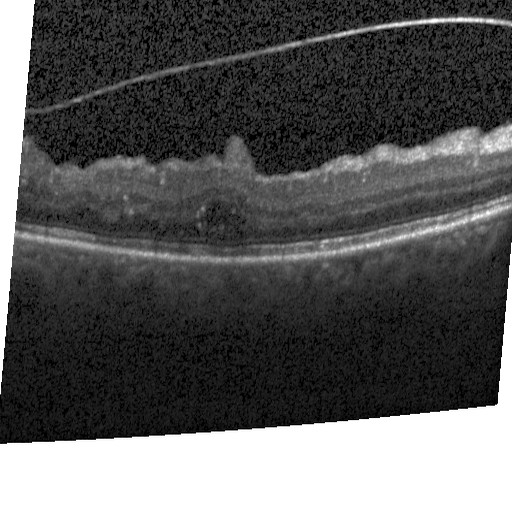
Impression: diabetic macular edema.